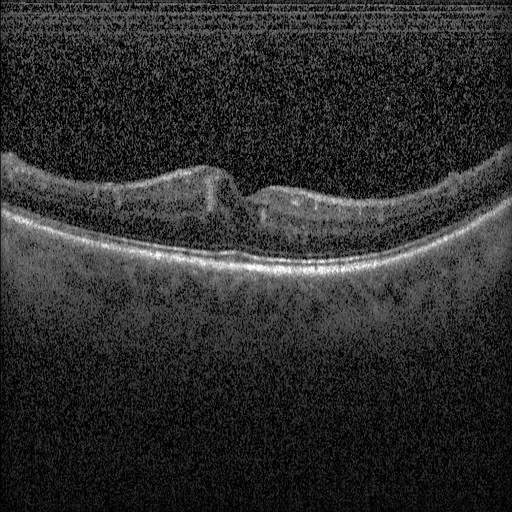
SD-OCT. OCT line scan. Heidelberg Spectralis
Impression: diabetic macular edema.